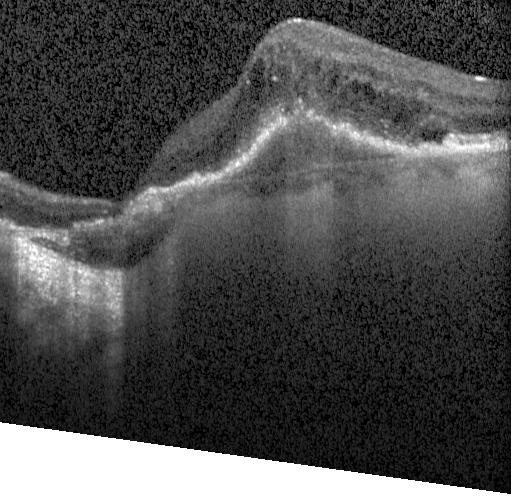 Optical coherence tomography B-scan.
Finding: CNV.